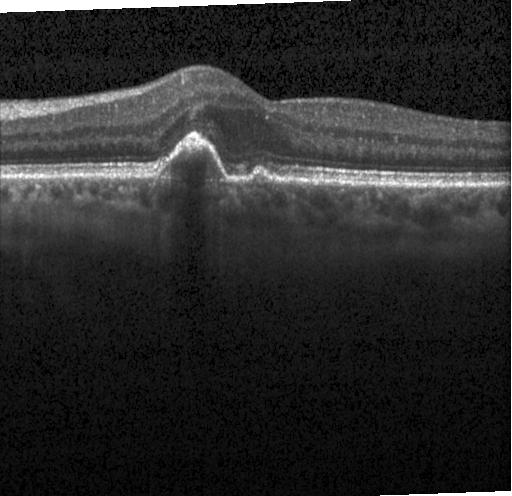
Instrument: Heidelberg Spectralis. SD-OCT. OCT line scan. OCT finding: a choroidal neovascular membrane.